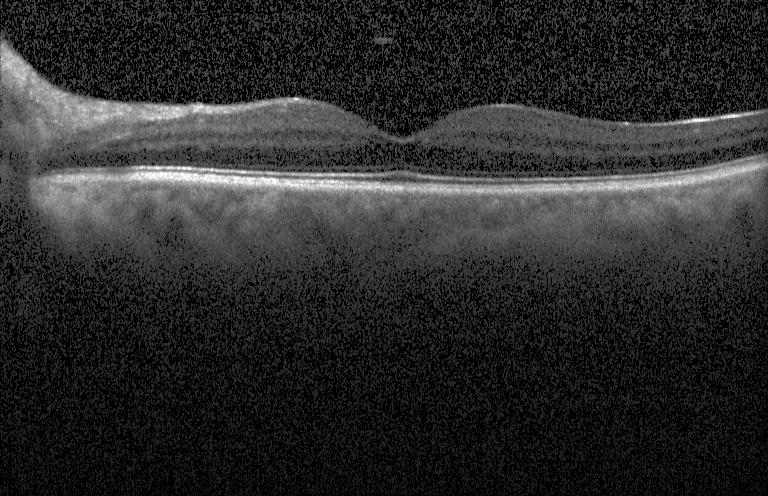
Retinal OCT cross-section. Impression: no choroidal neovascularization, diabetic macular edema, or drusen.